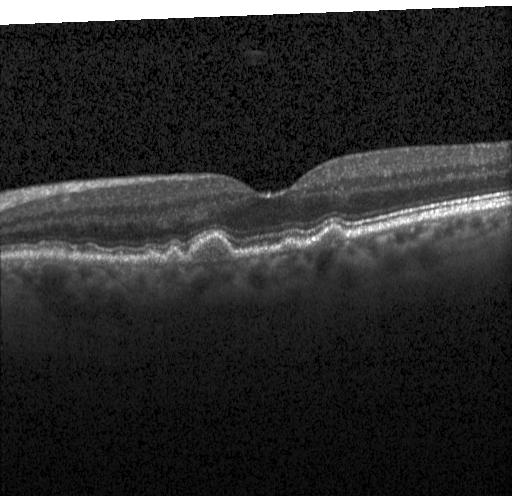
Impression: drusen.